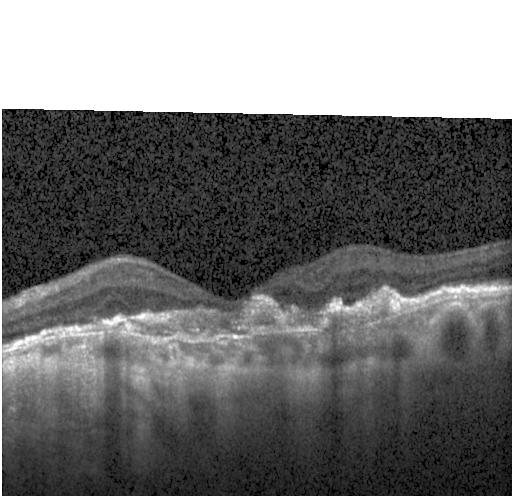
This B-scan demonstrates choroidal neovascularization.